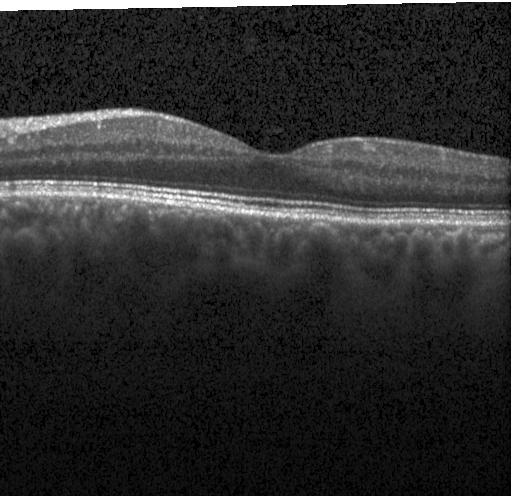
Assessment: neither choroidal neovascularization, diabetic macular edema, nor drusen.